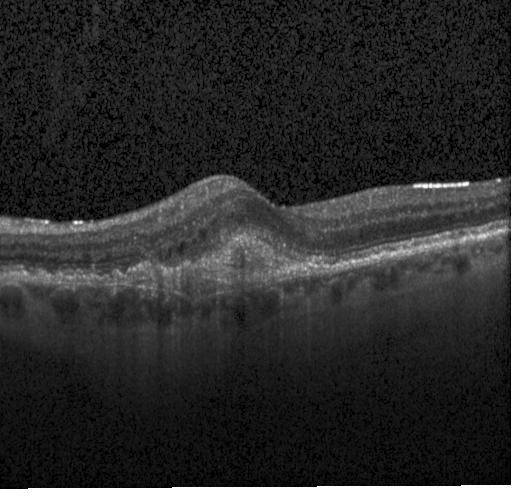
Heidelberg Spectralis; retinal OCT cross-section. OCT finding: a choroidal neovascular membrane.